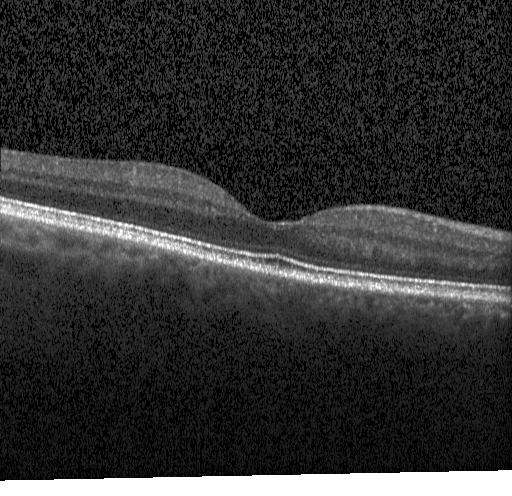

Spectral-domain OCT, Heidelberg Spectralis OCT system, optical coherence tomography B-scan, centered on the fovea — Impression: neither CNV, DME, nor drusen.